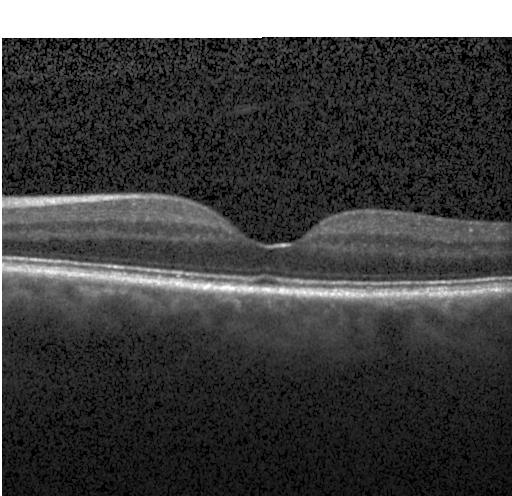

Horizontal scan through the fovea · instrument: Heidelberg Spectralis · OCT B-scan · spectral-domain optical coherence tomography.
Impression: no choroidal neovascularization, diabetic macular edema, or drusen.